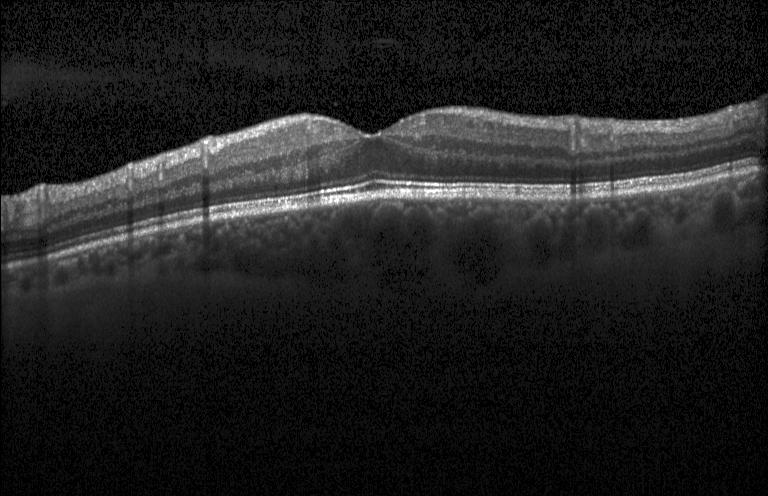
OCT B-scan.
Impression: no choroidal neovascularization, no diabetic macular edema, and no drusen.